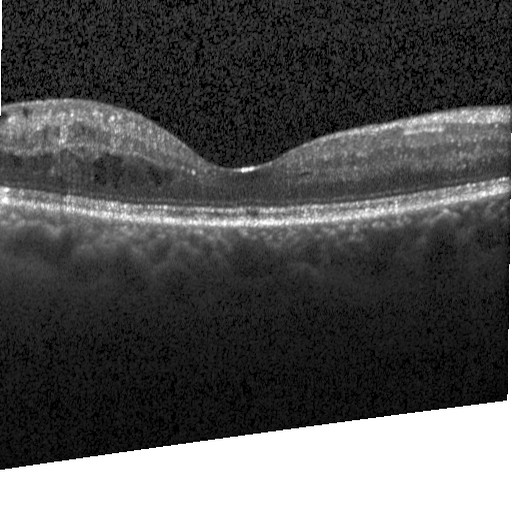

Retinal OCT cross-section; macular scan; acquired on a Heidelberg Spectralis — Impression: diabetic macular edema.